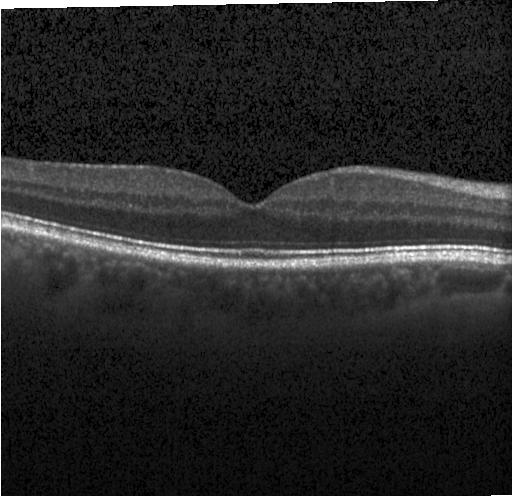
Acquired on a Heidelberg Spectralis · macular scan · optical coherence tomography scan
Diagnosis: no choroidal neovascularization, no diabetic macular edema, and no drusen.